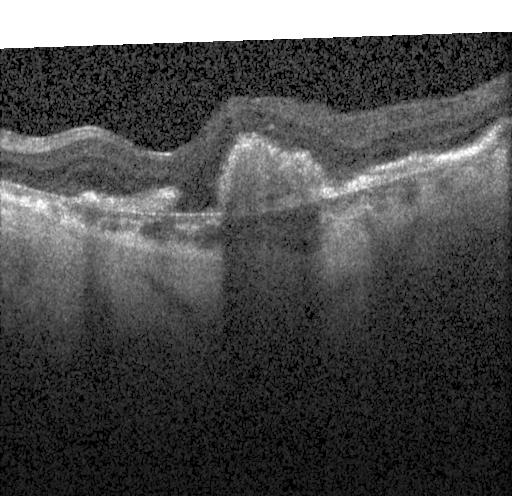
Spectral-domain OCT B-scan: CNV.